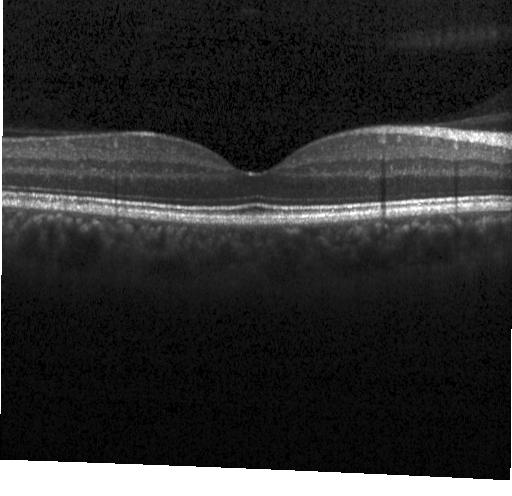 Diagnosis: no evidence of CNV, DME, or drusen.